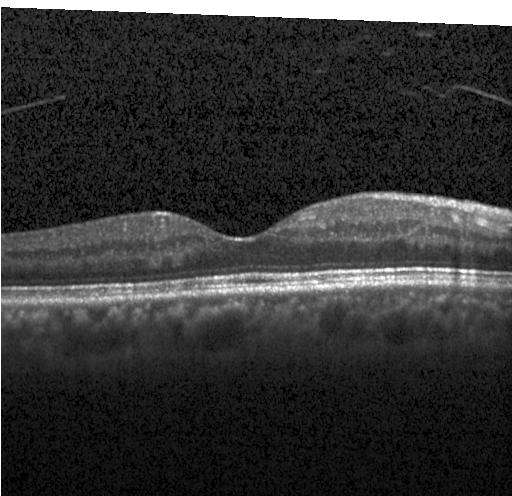

Dx: no choroidal neovascularization, diabetic macular edema, or drusen.